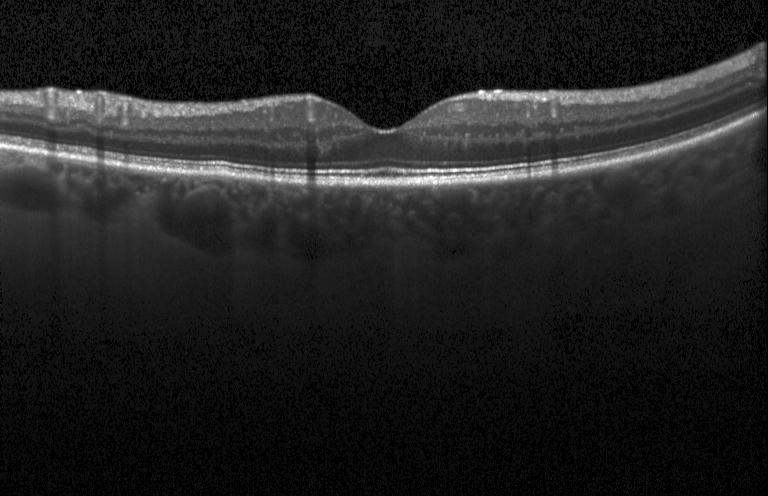

Optical coherence tomography scan. Through the macula — Macular OCT: no evidence of choroidal neovascularization, diabetic macular edema, or drusen.